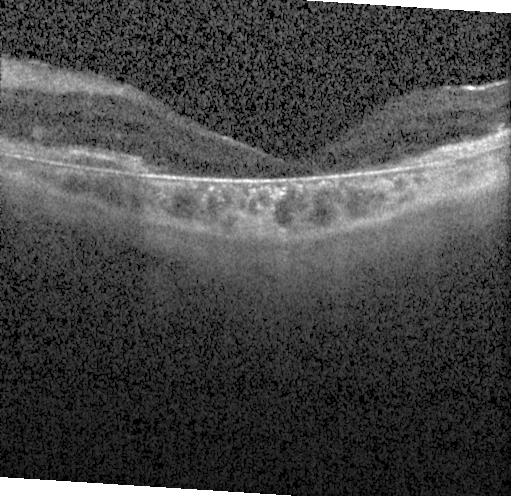 Spectral-domain optical coherence tomography. Horizontal scan through the fovea. Retinal OCT cross-section — Assessment: CNV.